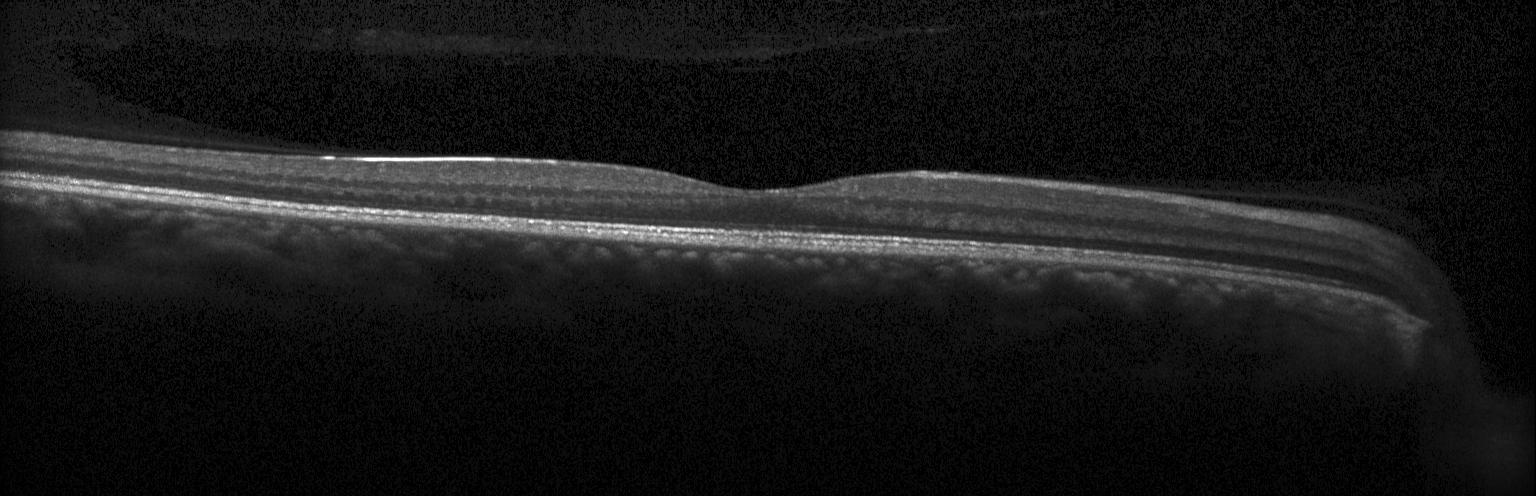 OCT scan showing neither choroidal neovascularization, diabetic macular edema, nor drusen.